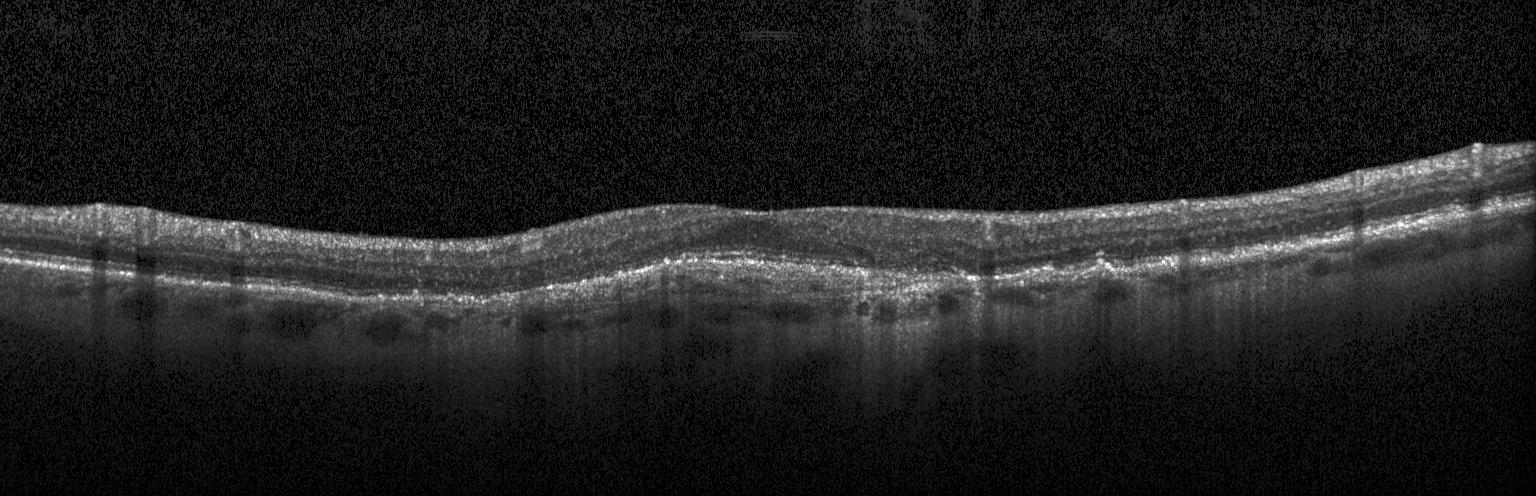

Optical coherence tomography B-scan.
Assessment: a choroidal neovascular membrane.